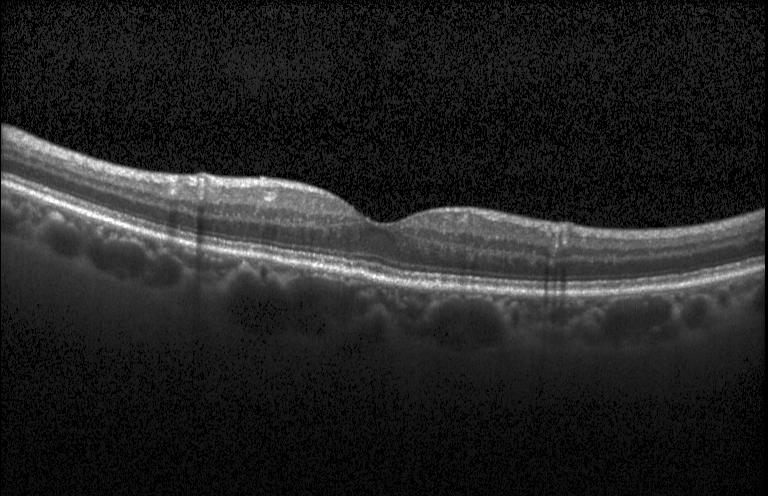
Spectral-domain OCT B-scan: no evidence of choroidal neovascularization, diabetic macular edema, or drusen.